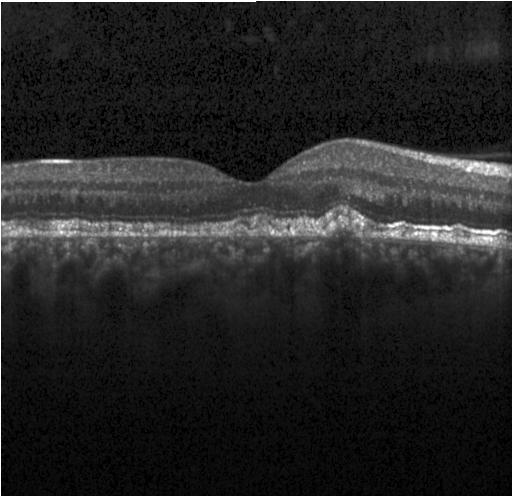
Instrument: Heidelberg Spectralis. SD-OCT. Macular scan. OCT line scan.
Finding: multiple drusen.